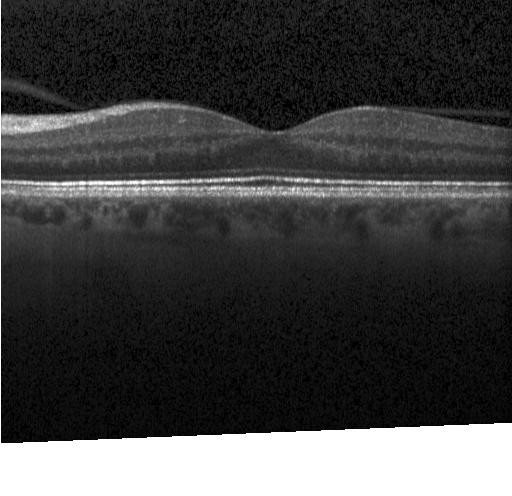

Heidelberg Spectralis. Optical coherence tomography B-scan. Spectral-domain OCT. Horizontal scan through the fovea. Macular OCT: no choroidal neovascularization, no diabetic macular edema, and no drusen.